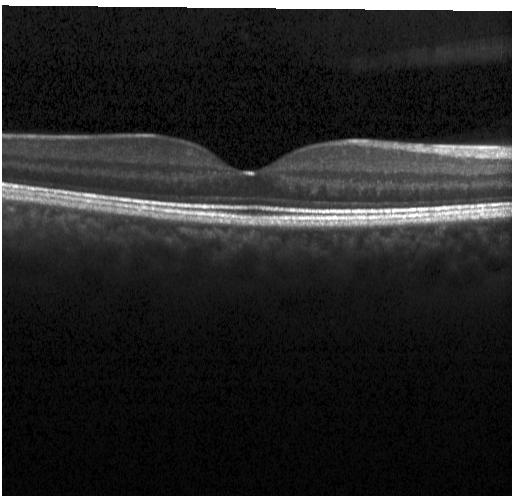 Retinal OCT B-scan, spectral-domain OCT, acquired on a Heidelberg Spectralis — Diagnosis: no choroidal neovascularization, diabetic macular edema, or drusen.